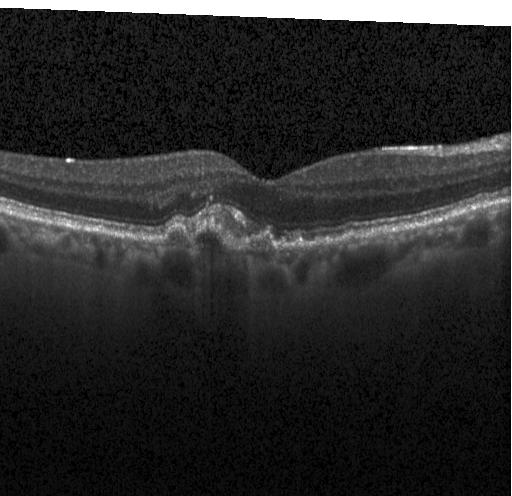
OCT line scan. Instrument: Heidelberg Spectralis — Diagnosis: choroidal neovascularization.